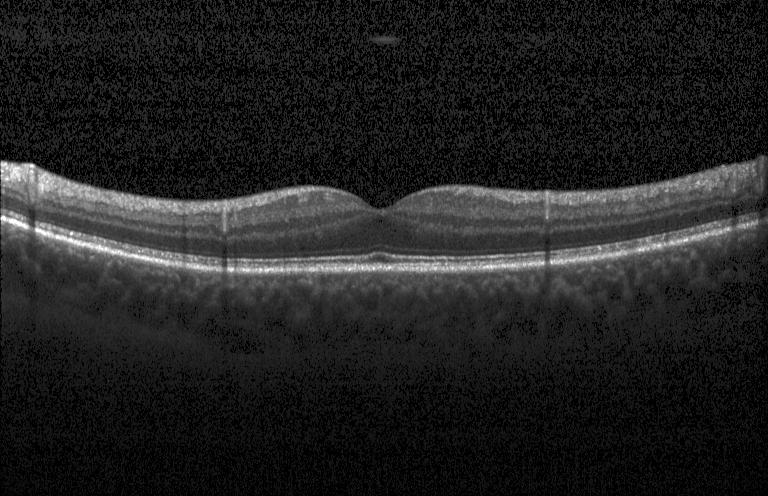

Retinal OCT B-scan.
This B-scan demonstrates no evidence of CNV, DME, or drusen.